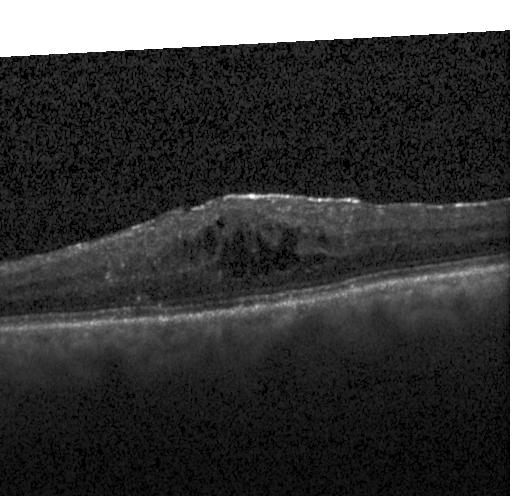 Diagnosis: DME.